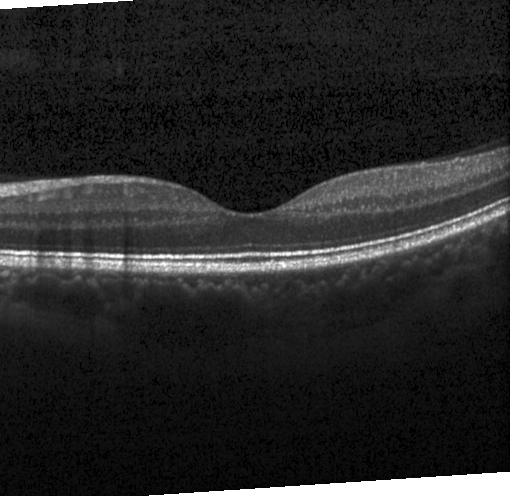
Spectral-domain optical coherence tomography · Heidelberg Spectralis OCT system · retinal OCT cross-section.
Dx: neither choroidal neovascularization, diabetic macular edema, nor drusen.